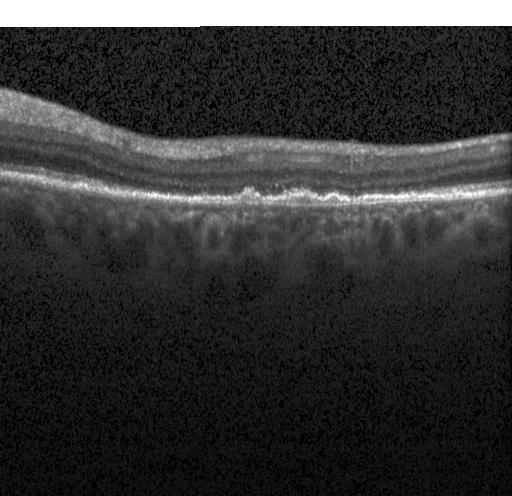
Retinal OCT cross-section showing a choroidal neovascular membrane.